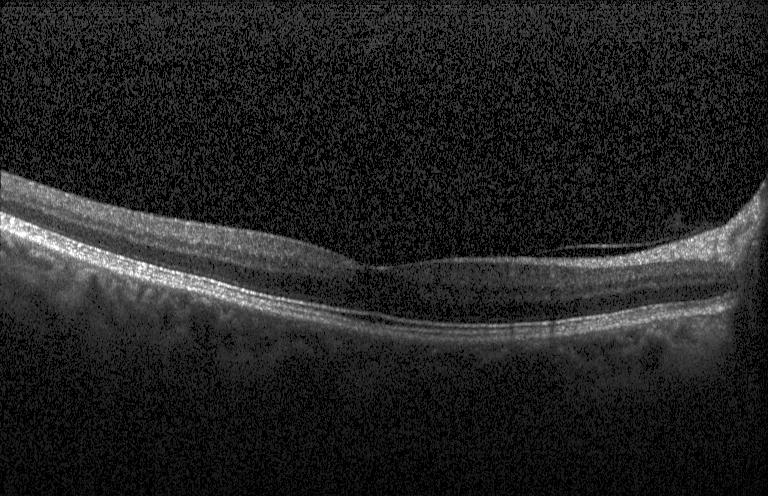

Optical coherence tomography scan, spectral-domain optical coherence tomography
Macular OCT: no choroidal neovascularization, diabetic macular edema, or drusen.